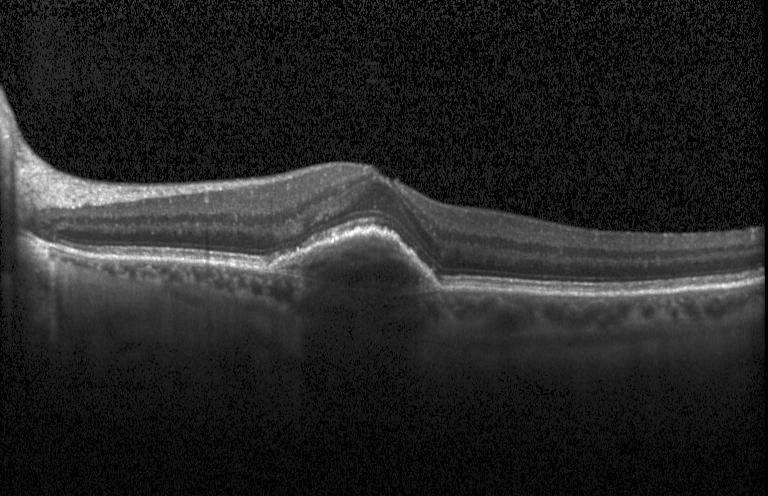

OCT B-scan
Finding: choroidal neovascularization.